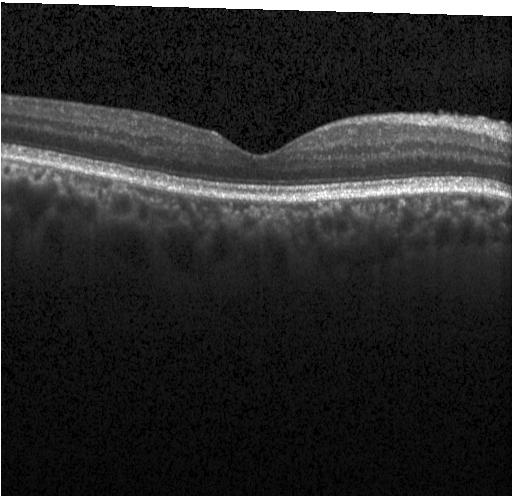

Centered on the fovea; optical coherence tomography B-scan.
Diagnosis: neither CNV, DME, nor drusen.